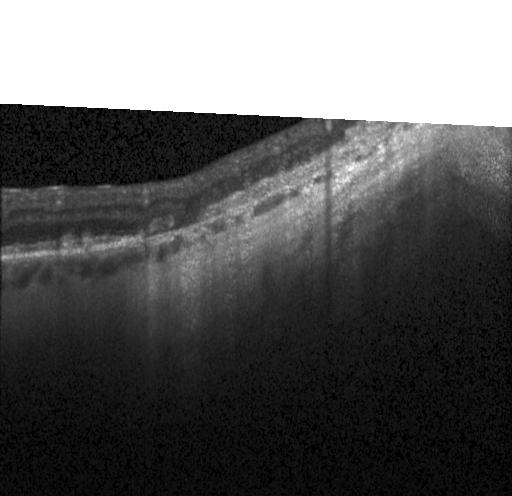

Retinal OCT cross-section showing choroidal neovascularization (CNV).